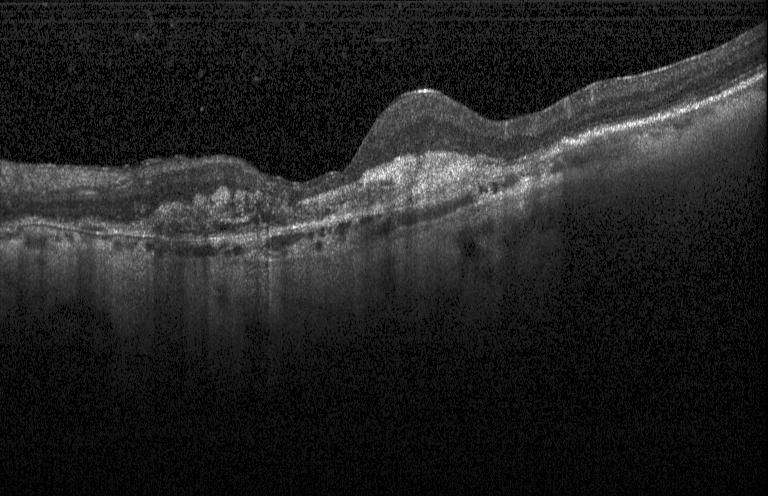

Finding: choroidal neovascularization.